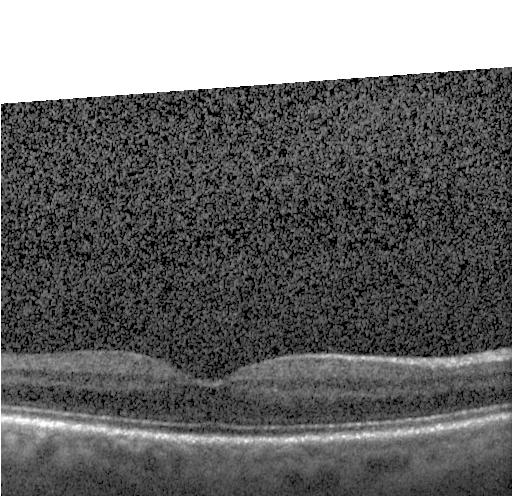

OCT line scan — Dx: no choroidal neovascularization, no diabetic macular edema, and no drusen.